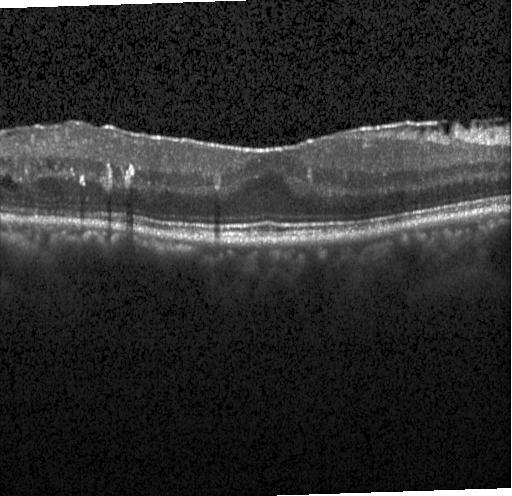

Centered on the fovea; acquired on a Heidelberg Spectralis; optical coherence tomography B-scan. Diagnosis: DME.